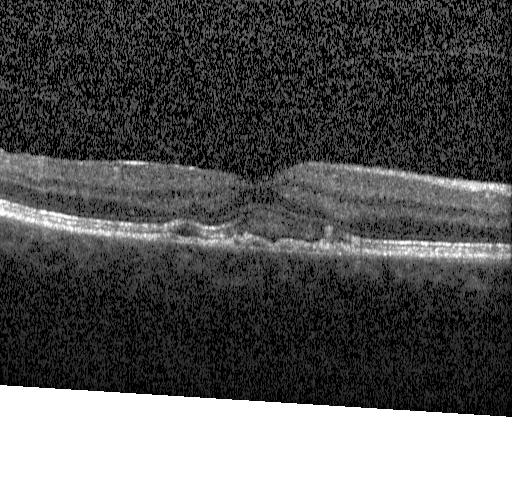
Optical coherence tomography scan. Impression: CNV.